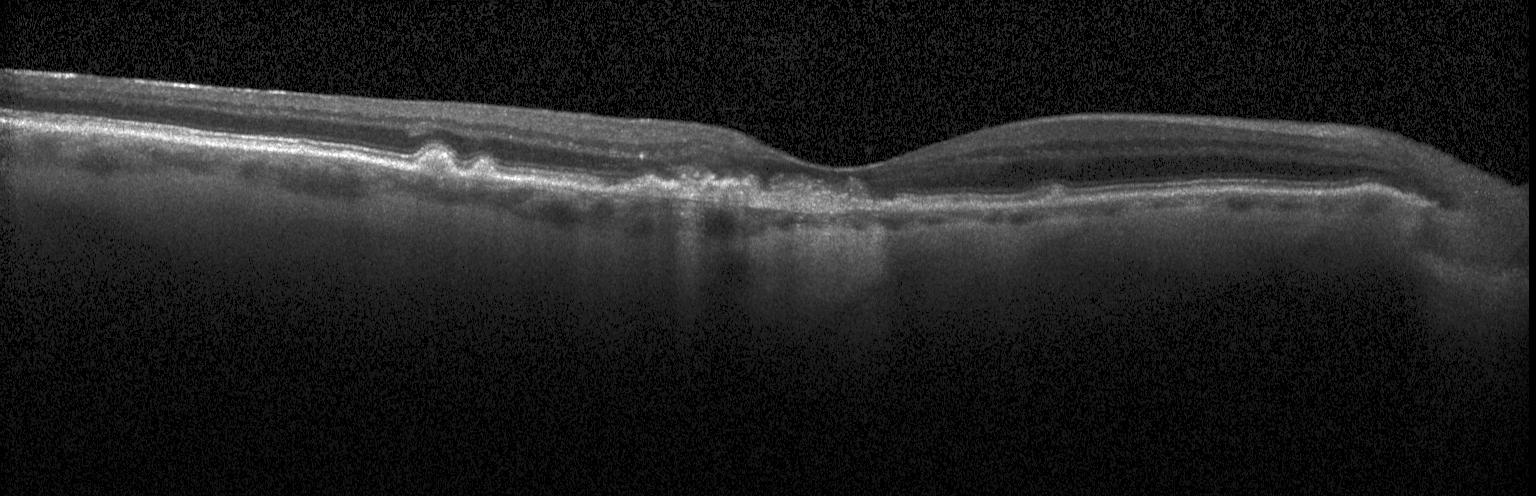 Spectral-domain optical coherence tomography, Heidelberg Spectralis, macular scan, optical coherence tomography scan — Dx: a choroidal neovascular membrane.